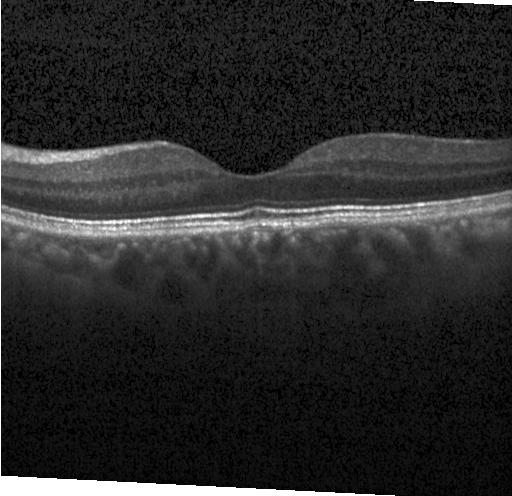
SD-OCT; retinal OCT B-scan; horizontal scan through the fovea. Macular OCT: no choroidal neovascularization, diabetic macular edema, or drusen.